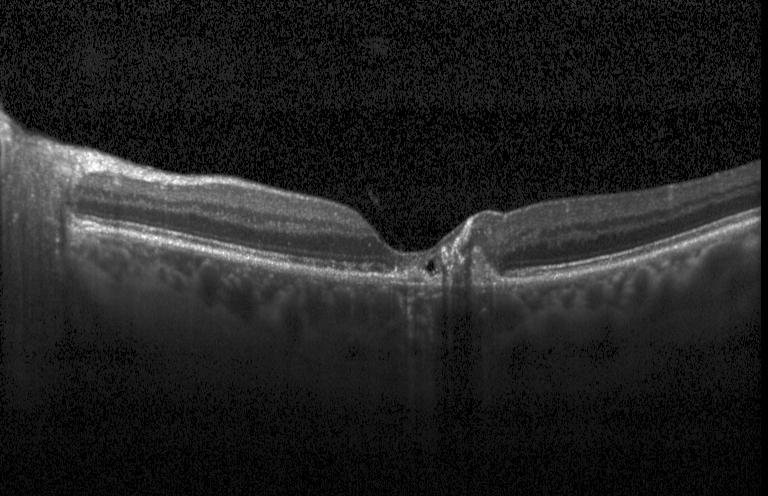 Retinal OCT cross-section showing a choroidal neovascular membrane.